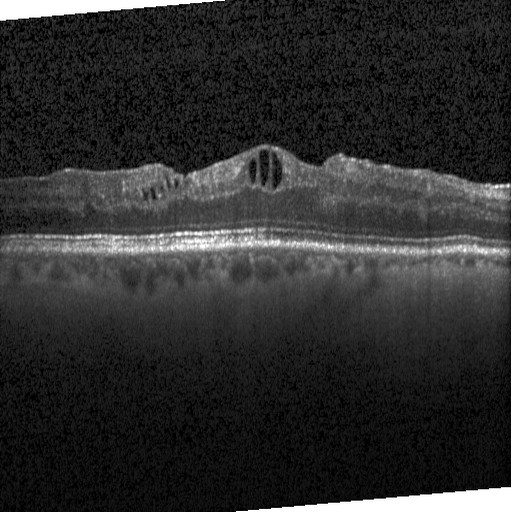 Spectral-domain OCT B-scan: diabetic macular edema.